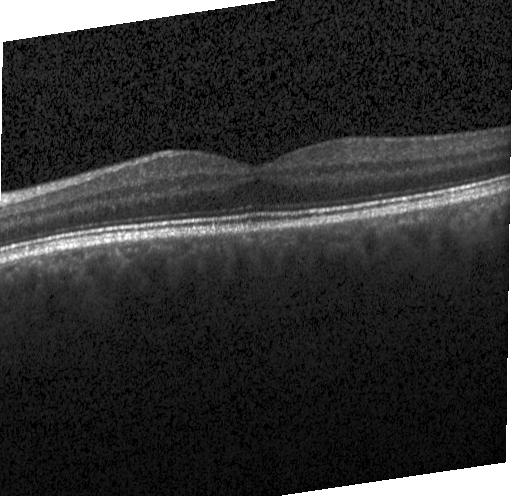
Through the macula; optical coherence tomography scan; instrument: Heidelberg Spectralis; spectral-domain optical coherence tomography. Dx: no choroidal neovascularization, diabetic macular edema, or drusen.